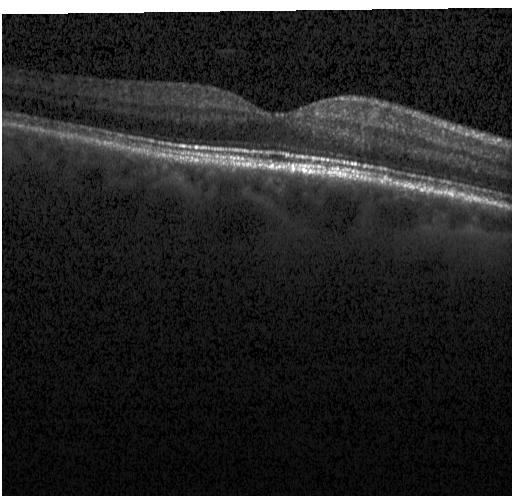
Assessment: neither choroidal neovascularization, diabetic macular edema, nor drusen.